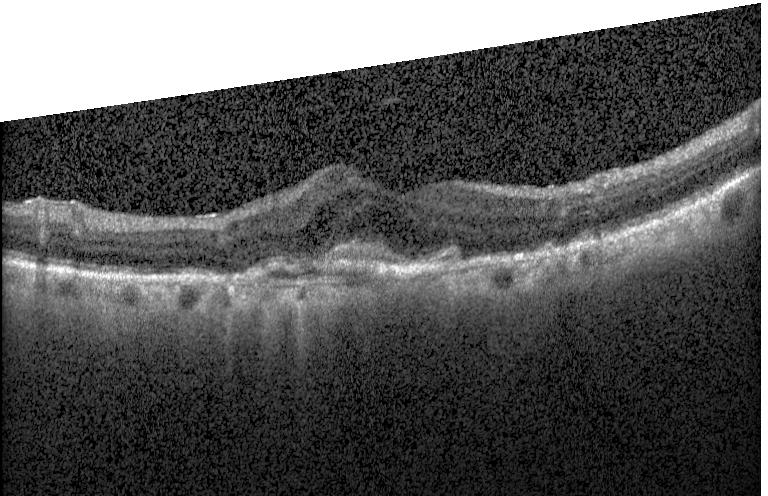

OCT B-scan. Horizontal scan through the fovea. SD-OCT — Impression: a choroidal neovascular membrane.